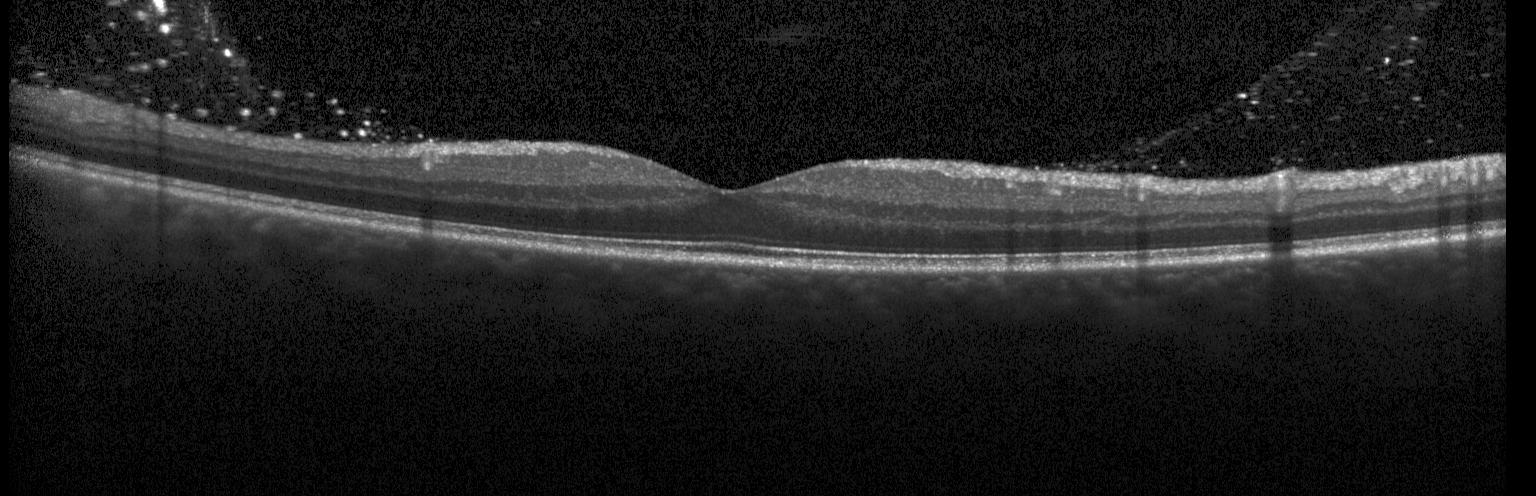 SD-OCT; optical coherence tomography scan.
This B-scan demonstrates no evidence of choroidal neovascularization, diabetic macular edema, or drusen.